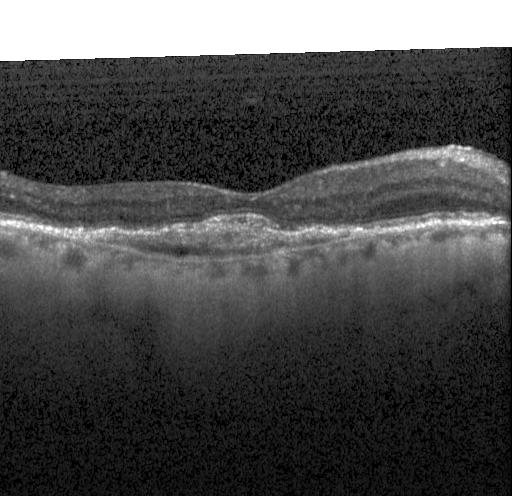
Spectral-domain OCT · optical coherence tomography B-scan
This B-scan demonstrates choroidal neovascularization (CNV).